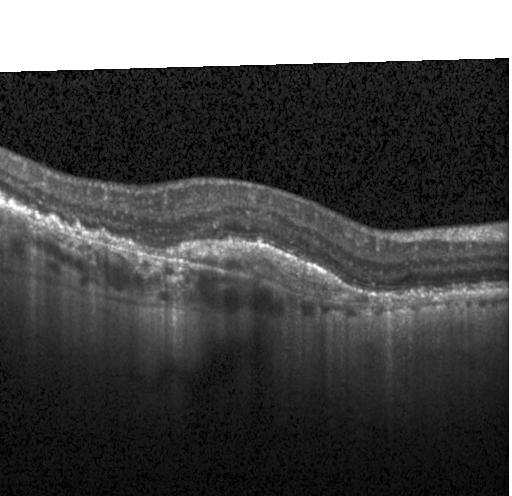
Dx: a choroidal neovascular membrane.